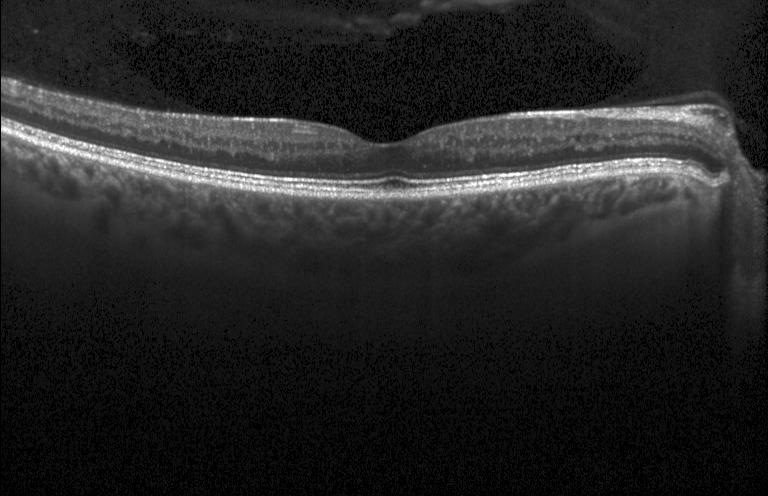
Retinal OCT cross-section. No evidence of CNV, DME, or drusen.